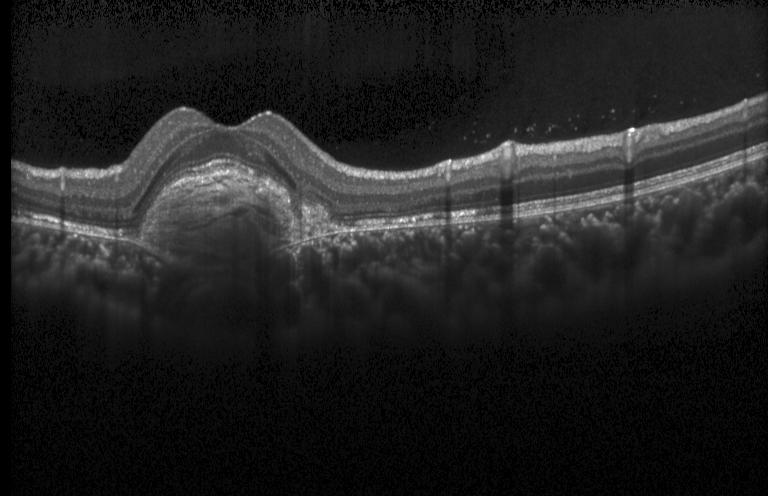
Retinal OCT cross-section showing choroidal neovascularization.